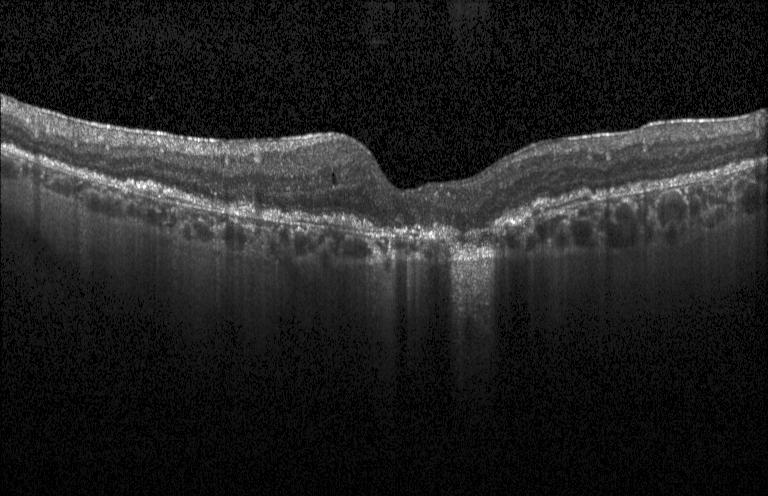

OCT finding: a choroidal neovascular membrane.